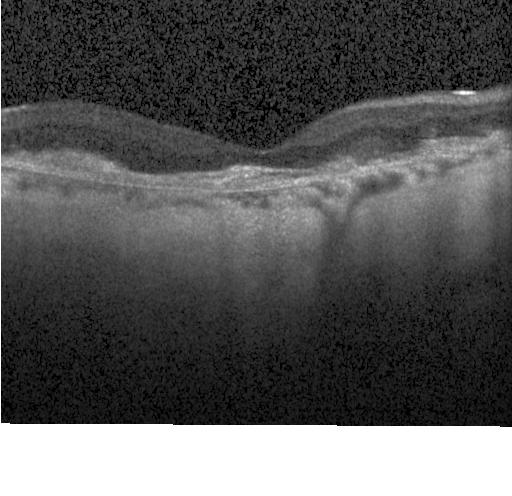

Retinal OCT cross-section. OCT finding: a choroidal neovascular membrane.